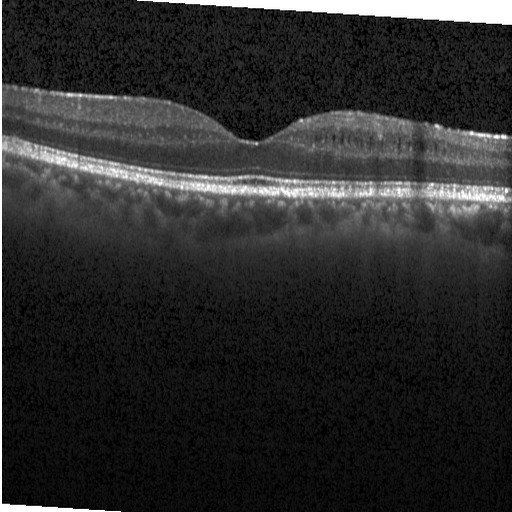
SD-OCT, through the macula, instrument: Heidelberg Spectralis, OCT line scan. This B-scan demonstrates DME.